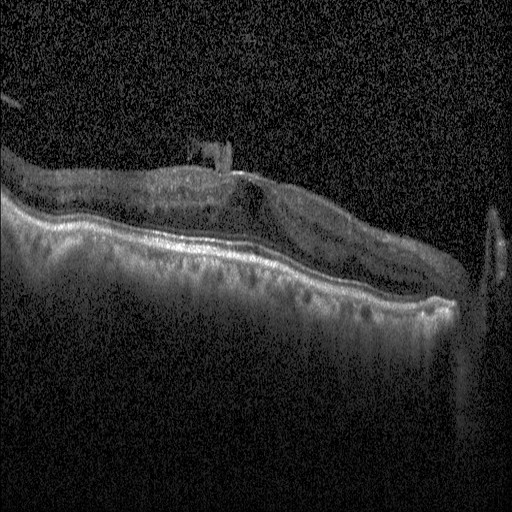 OCT B-scan · fovea-centered · spectral-domain optical coherence tomography · instrument: Heidelberg Spectralis — Diabetic macular edema (DME).